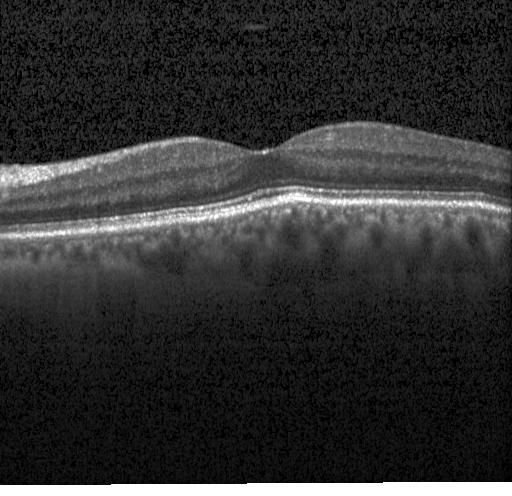

Heidelberg Spectralis OCT system · optical coherence tomography B-scan
Finding: no evidence of CNV, DME, or drusen.